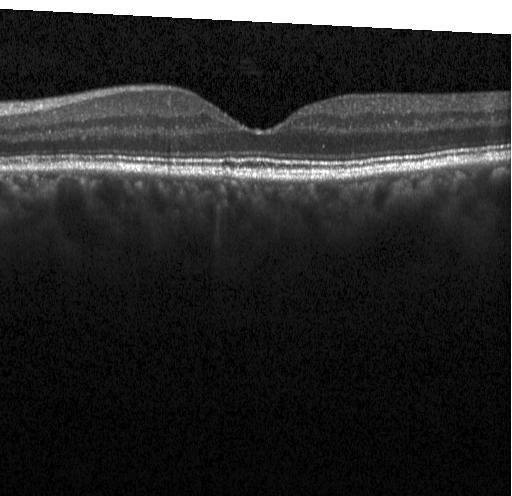

Retinal OCT cross-section showing no evidence of choroidal neovascularization, diabetic macular edema, or drusen.